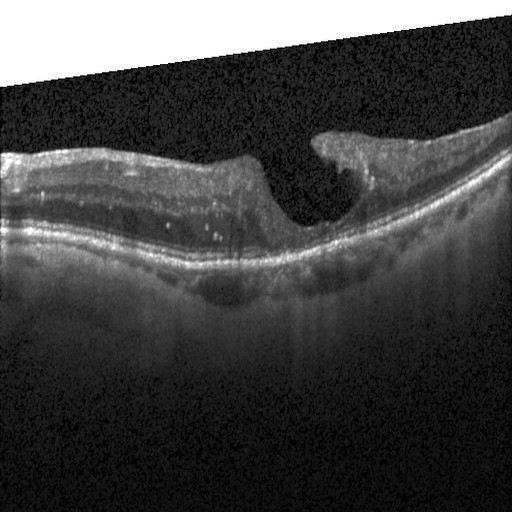 Horizontal scan through the fovea · Heidelberg Spectralis · optical coherence tomography B-scan — This B-scan demonstrates DME.